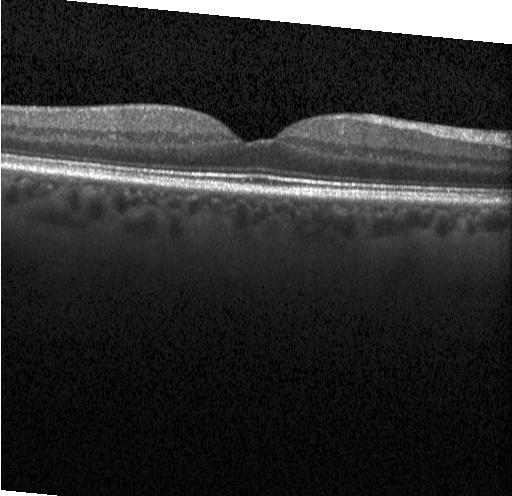
SD-OCT, OCT line scan, through the macula
Assessment: neither choroidal neovascularization, diabetic macular edema, nor drusen.